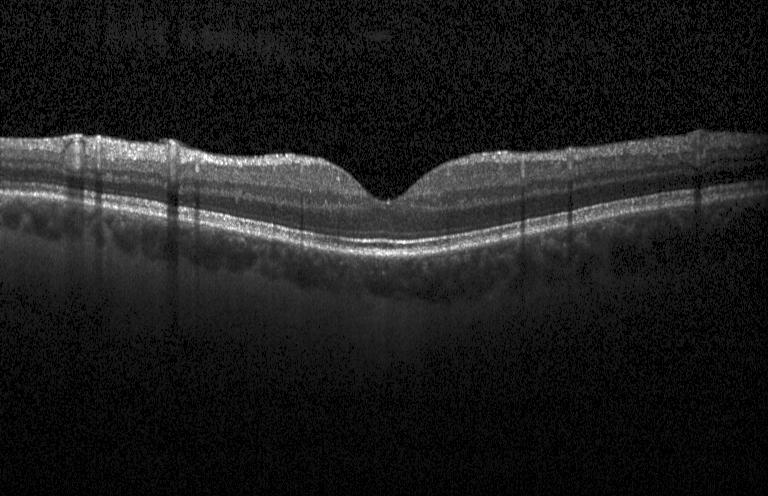 Heidelberg Spectralis · retinal OCT B-scan · spectral-domain OCT — OCT finding: no evidence of CNV, DME, or drusen.